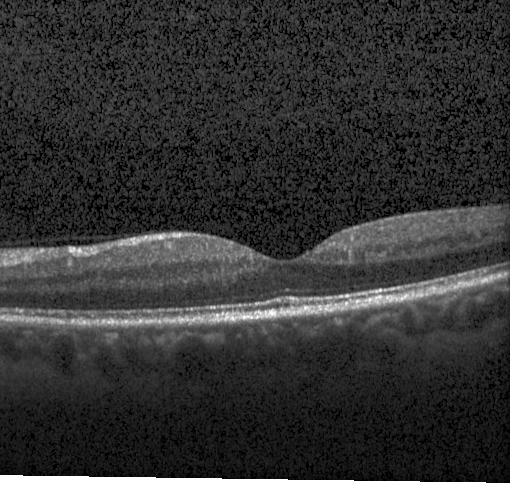
Spectral-domain OCT, optical coherence tomography B-scan, Heidelberg Spectralis, fovea-centered. The scan shows no choroidal neovascularization, diabetic macular edema, or drusen.